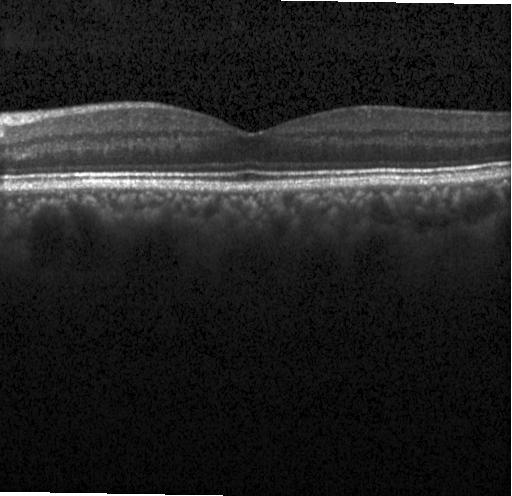 OCT B-scan.
Diagnosis: no choroidal neovascularization, diabetic macular edema, or drusen.